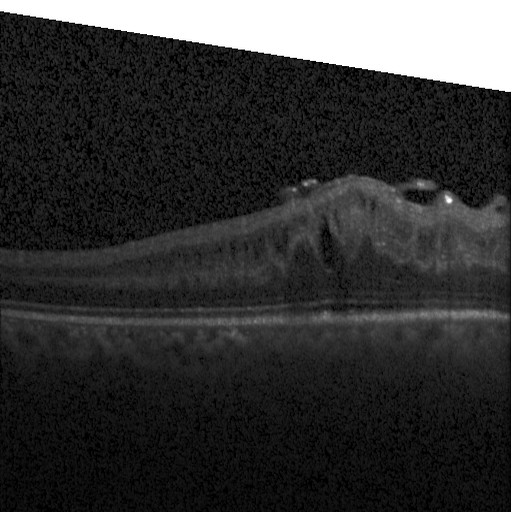

Fovea-centered, Heidelberg Spectralis OCT system, optical coherence tomography scan. Diagnosis: DME.